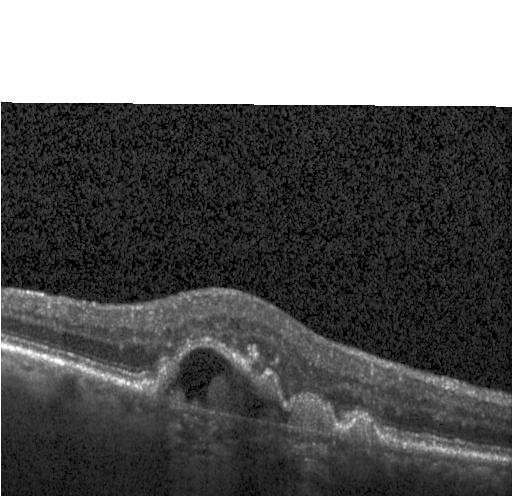
Optical coherence tomography B-scan · instrument: Heidelberg Spectralis.
Finding: a choroidal neovascular membrane.